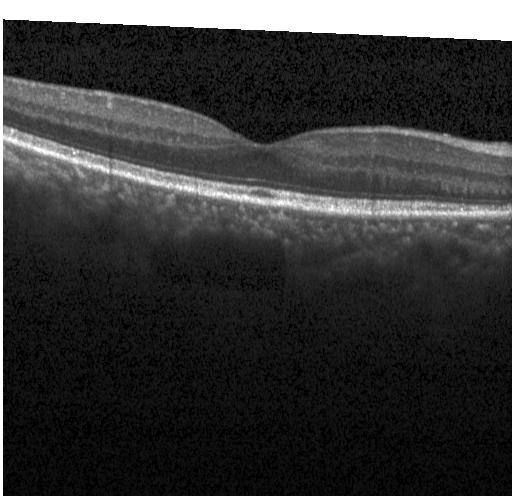 Acquired on a Heidelberg Spectralis; fovea-centered; OCT line scan; spectral-domain optical coherence tomography — Dx: no choroidal neovascularization, diabetic macular edema, or drusen.